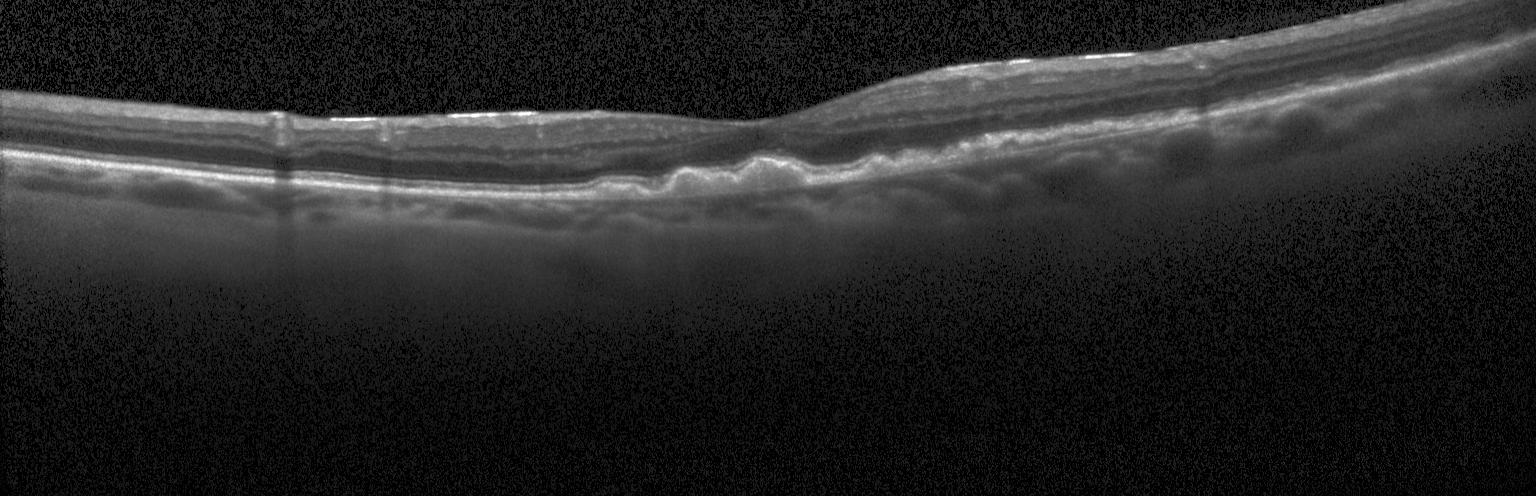
OCT finding: sub-RPE drusenoid deposits.